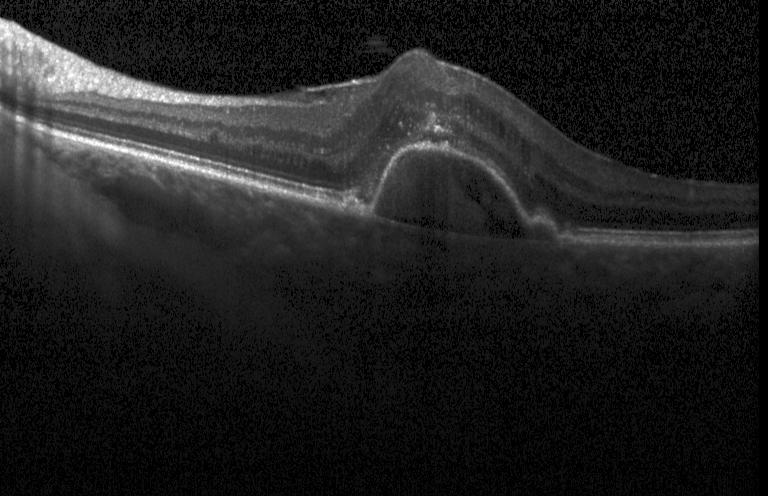 SD-OCT, centered on the fovea, retinal OCT B-scan — OCT finding: choroidal neovascularization (CNV).